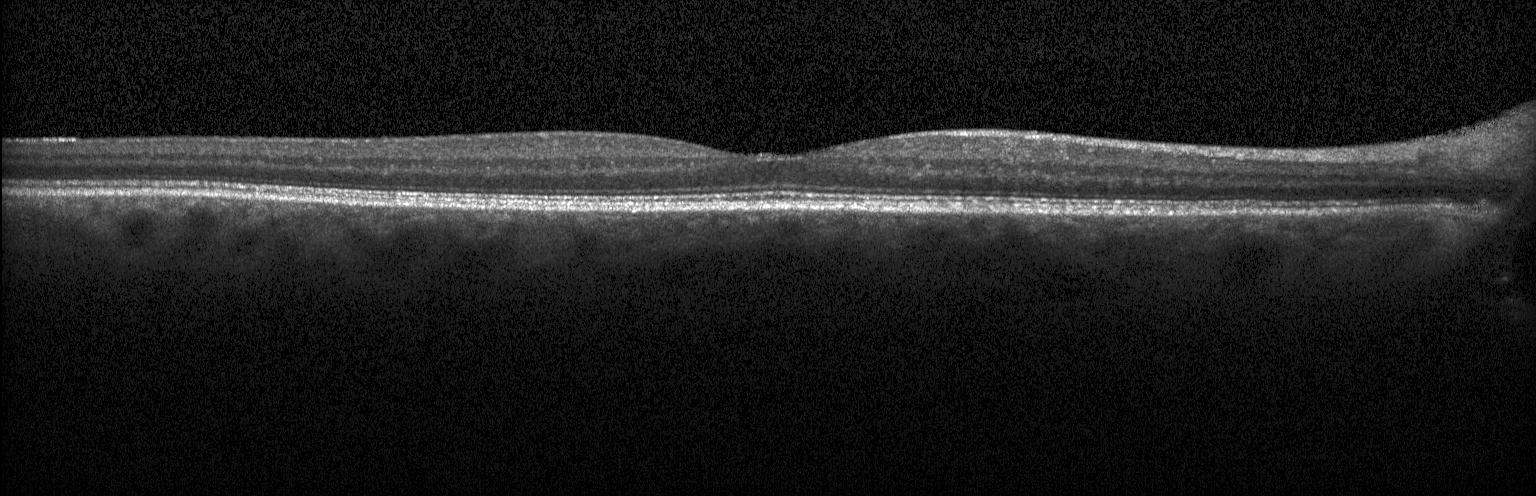
Retinal OCT cross-section, spectral-domain optical coherence tomography — Diagnosis: no evidence of CNV, DME, or drusen.